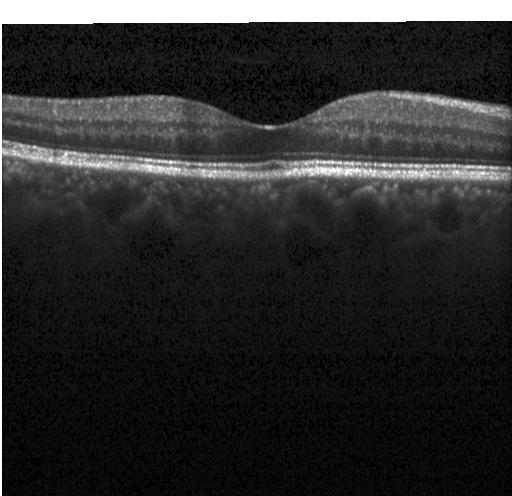
Spectral-domain OCT · OCT line scan — Diagnosis: neither CNV, DME, nor drusen.